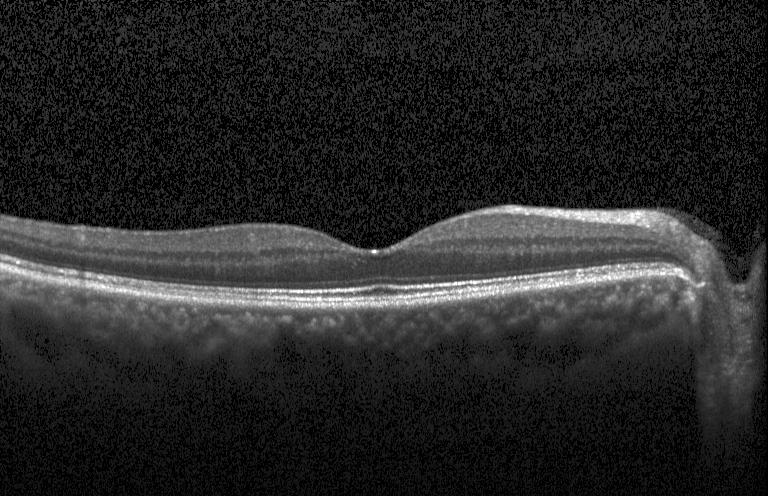
Optical coherence tomography B-scan. Impression: no CNV, no DME, and no drusen.